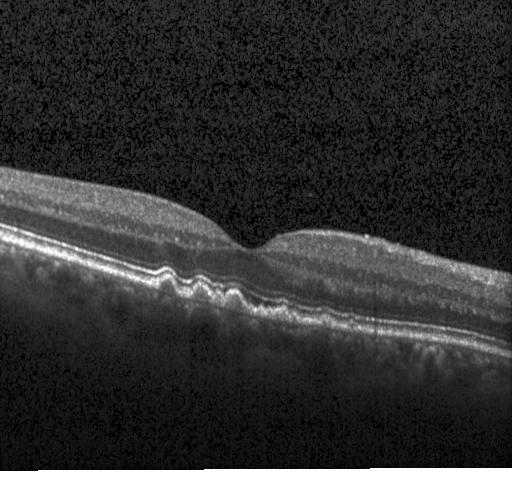 OCT B-scan
Finding: multiple drusen.